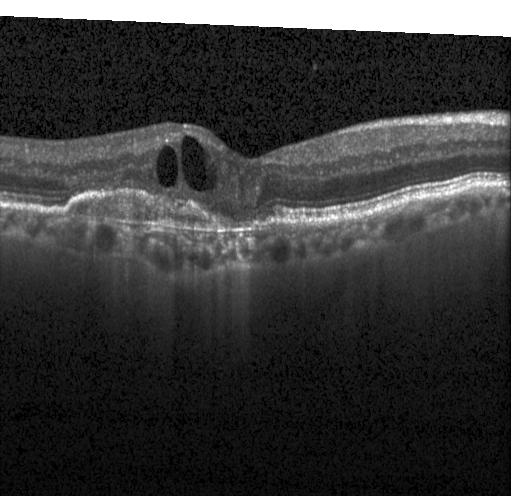
OCT line scan. Instrument: Heidelberg Spectralis — Diagnosis: CNV.